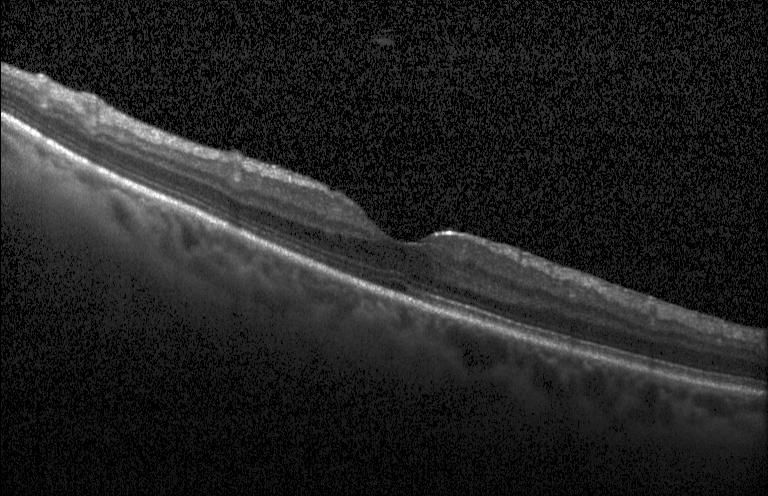
Assessment: neither CNV, DME, nor drusen.